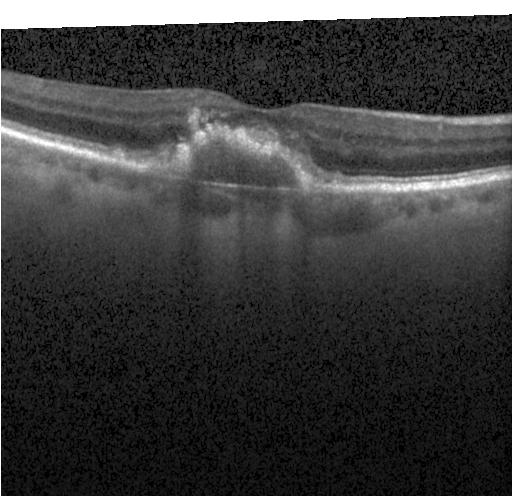 Heidelberg Spectralis OCT system, retinal OCT B-scan, spectral-domain optical coherence tomography — Assessment: a choroidal neovascular membrane.